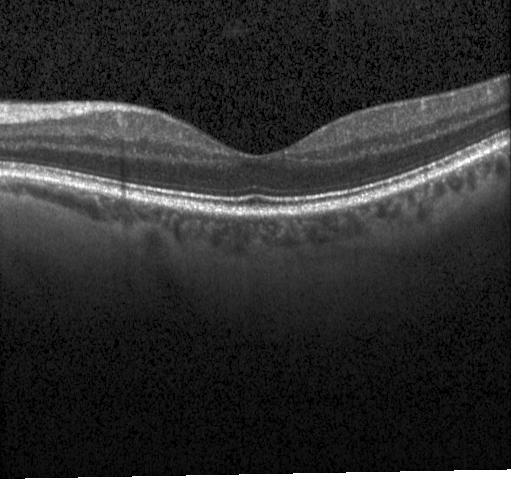 Optical coherence tomography B-scan · macular scan · SD-OCT · acquired on a Heidelberg Spectralis
Finding: no choroidal neovascularization, diabetic macular edema, or drusen.